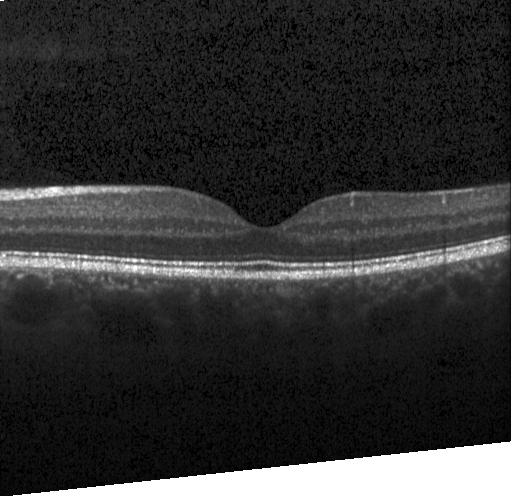 Spectral-domain OCT B-scan: neither choroidal neovascularization, diabetic macular edema, nor drusen.